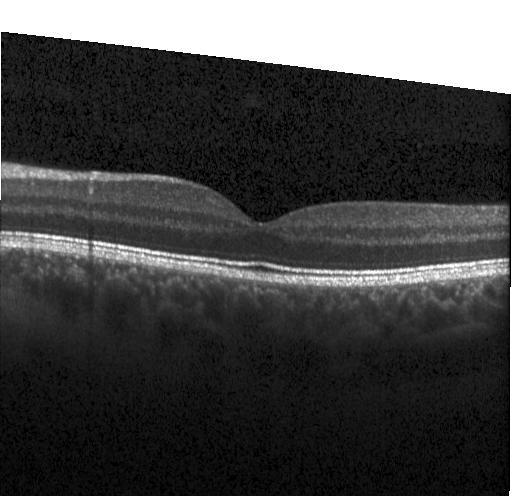 Finding: neither CNV, DME, nor drusen.